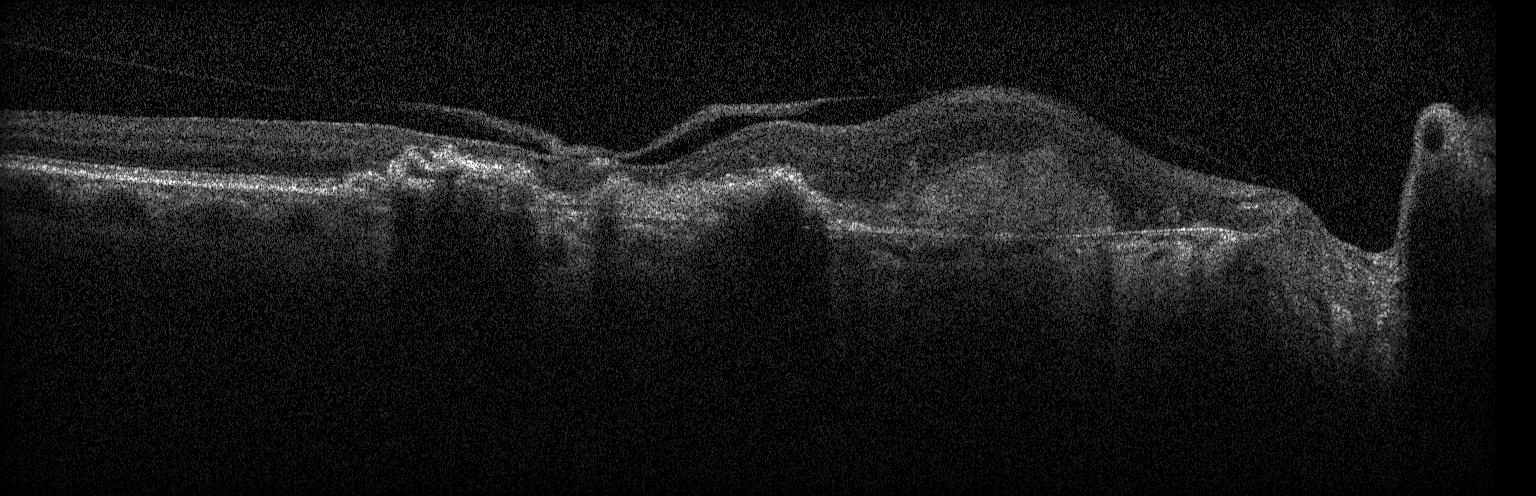

Instrument: Heidelberg Spectralis. Centered on the fovea. SD-OCT. Optical coherence tomography scan — Finding: choroidal neovascularization.